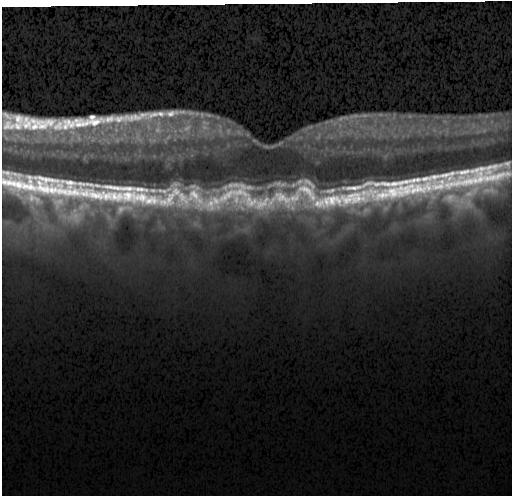

Optical coherence tomography B-scan, SD-OCT, acquired on a Heidelberg Spectralis, macular scan. Impression: multiple drusen.